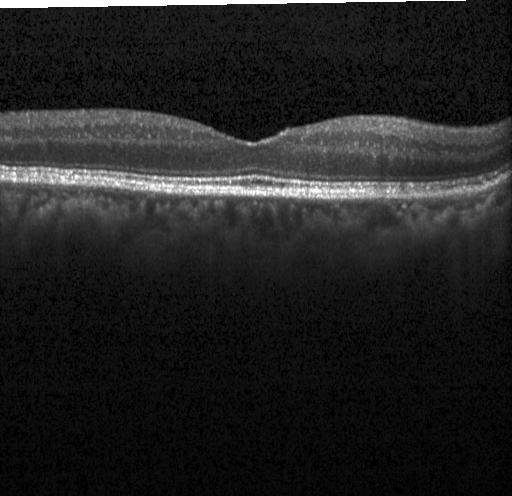

OCT finding: no evidence of choroidal neovascularization, diabetic macular edema, or drusen.